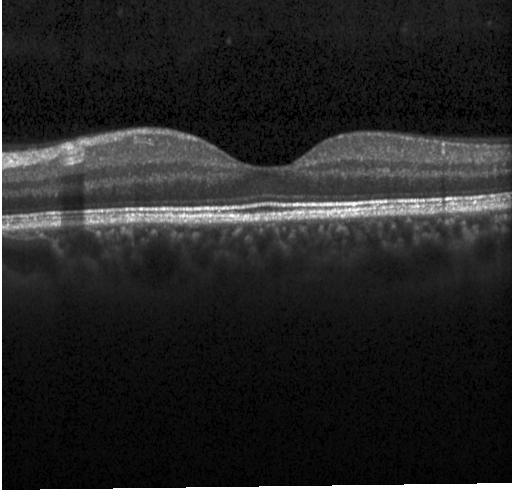 SD-OCT · macular scan · OCT line scan
Diagnosis: no evidence of CNV, DME, or drusen.